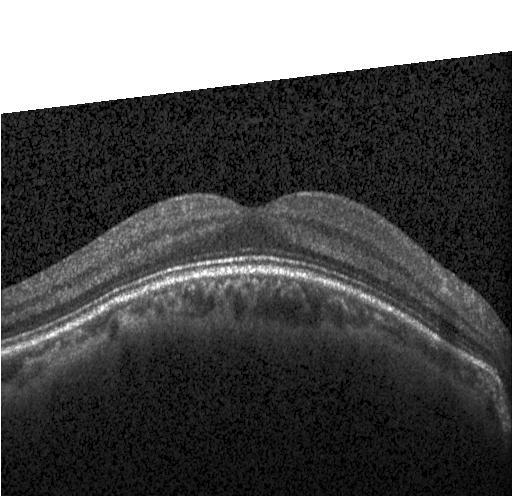 Retinal OCT B-scan; horizontal scan through the fovea. Impression: no evidence of choroidal neovascularization, diabetic macular edema, or drusen.